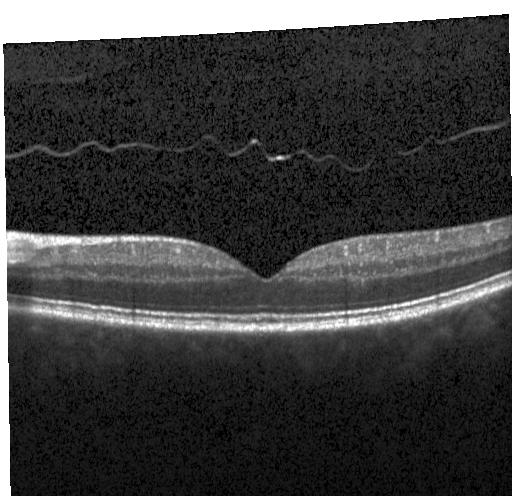
The scan shows neither choroidal neovascularization, diabetic macular edema, nor drusen.